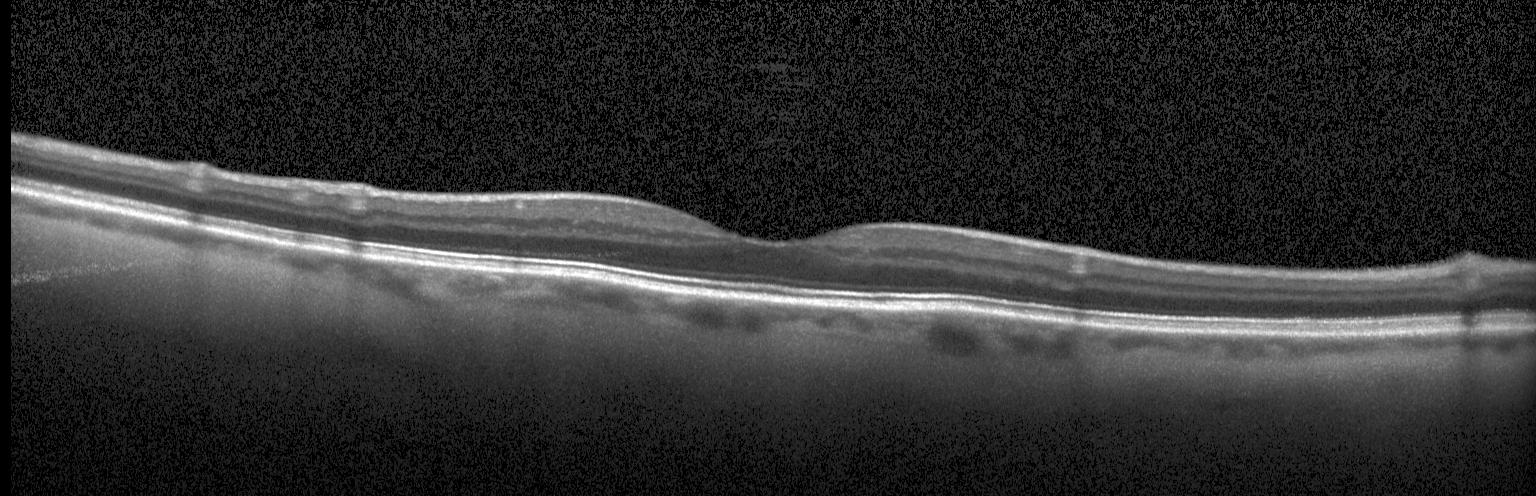

The scan shows no choroidal neovascularization, no diabetic macular edema, and no drusen.